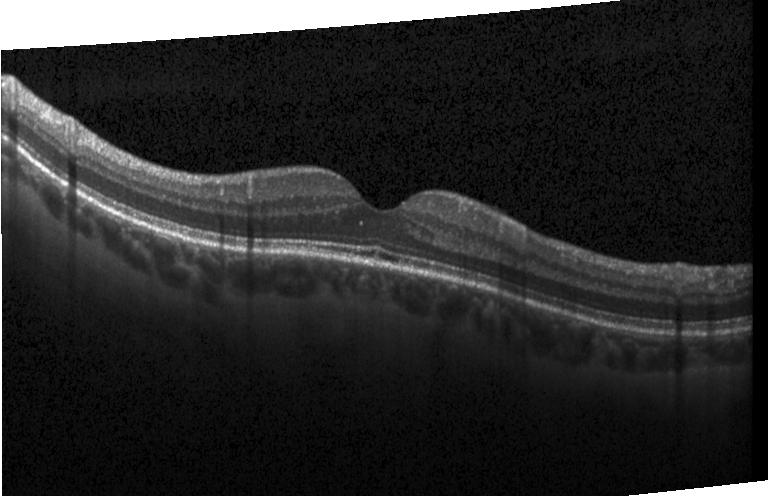

Acquired on a Heidelberg Spectralis. Spectral-domain OCT. Retinal OCT cross-section.
Finding: no choroidal neovascularization, no diabetic macular edema, and no drusen.